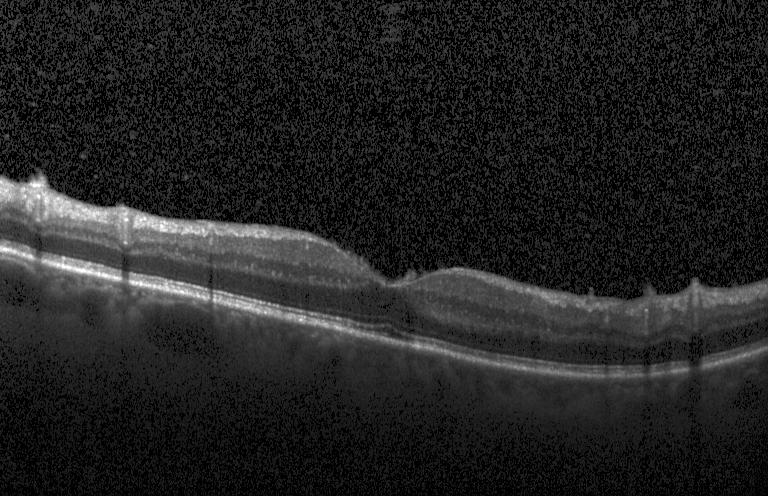
Assessment: no CNV, DME, or drusen.